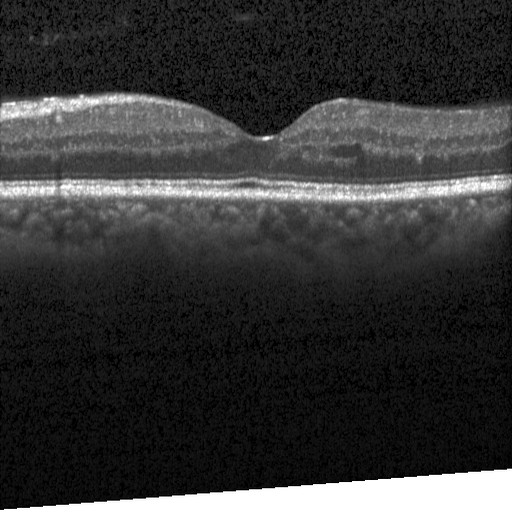 Retinal OCT cross-section · SD-OCT — Finding: DME.